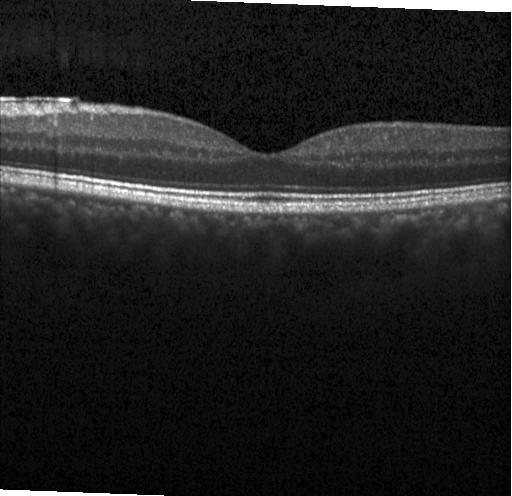
Macular scan · instrument: Heidelberg Spectralis · retinal OCT cross-section.
Impression: no evidence of CNV, DME, or drusen.